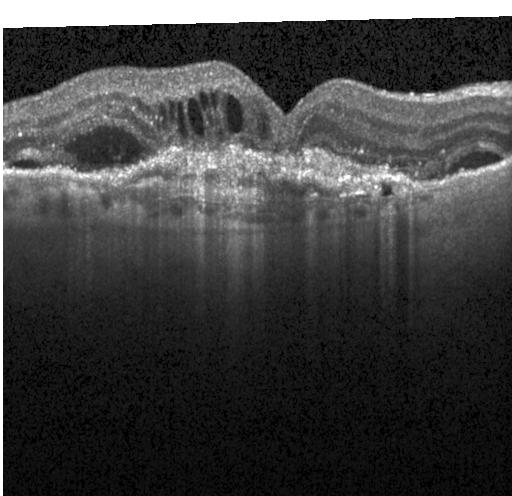
Retinal OCT cross-section · acquired on a Heidelberg Spectralis — Dx: a choroidal neovascular membrane.